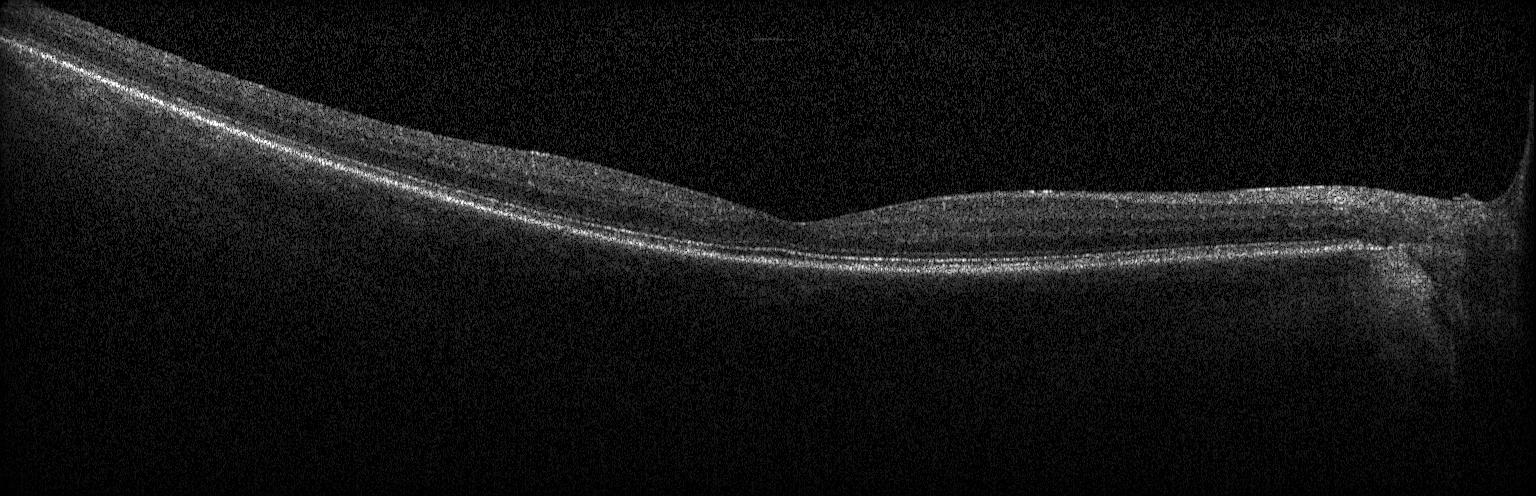 Instrument: Heidelberg Spectralis, retinal OCT cross-section, SD-OCT, horizontal scan through the fovea — This B-scan demonstrates no CNV, DME, or drusen.